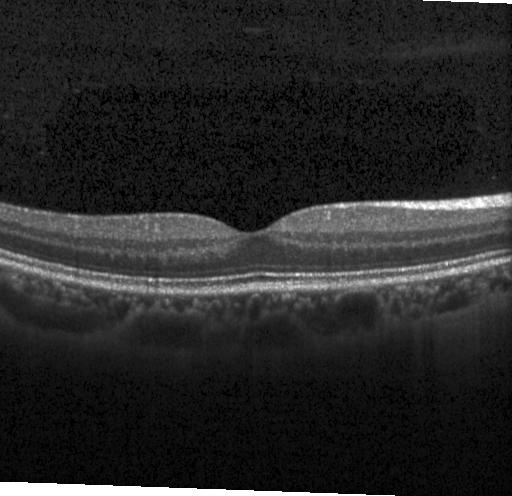
Finding: neither choroidal neovascularization, diabetic macular edema, nor drusen.